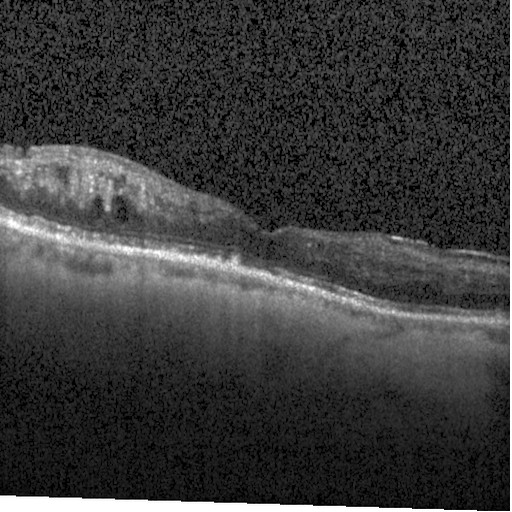

OCT B-scan showing diabetic macular edema (DME).